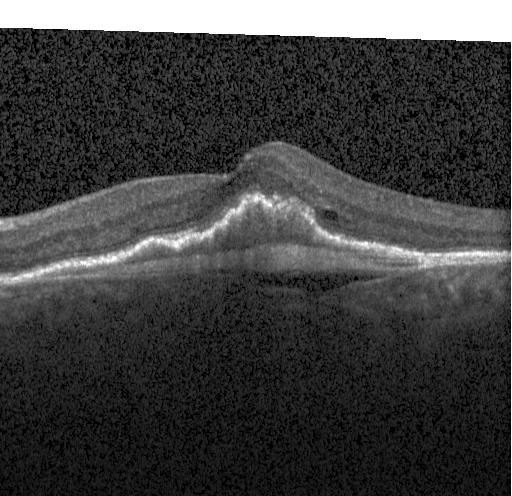 Acquired on a Heidelberg Spectralis; spectral-domain optical coherence tomography; OCT line scan
OCT finding: a choroidal neovascular membrane.